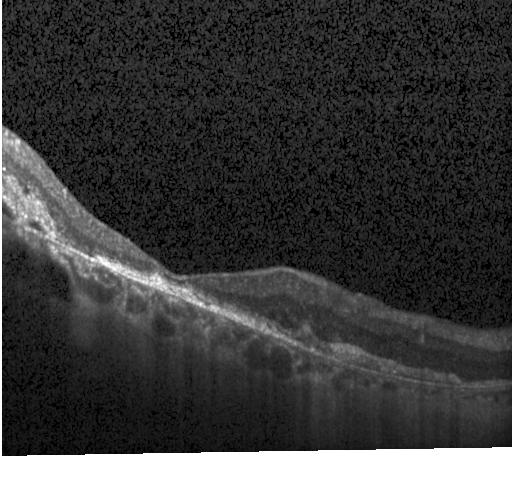
Optical coherence tomography B-scan — Diagnosis: a choroidal neovascular membrane.